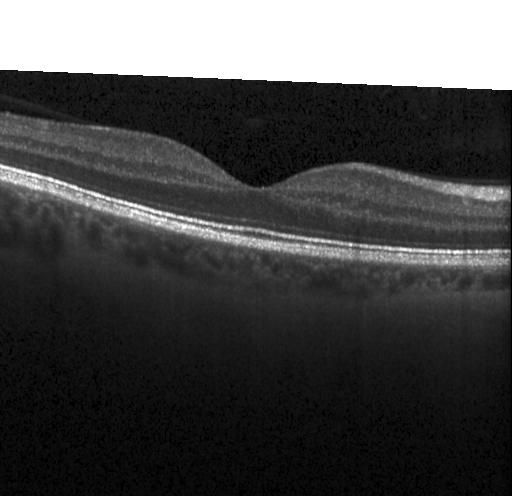
OCT line scan, fovea-centered, spectral-domain OCT.
Finding: no choroidal neovascularization, no diabetic macular edema, and no drusen.